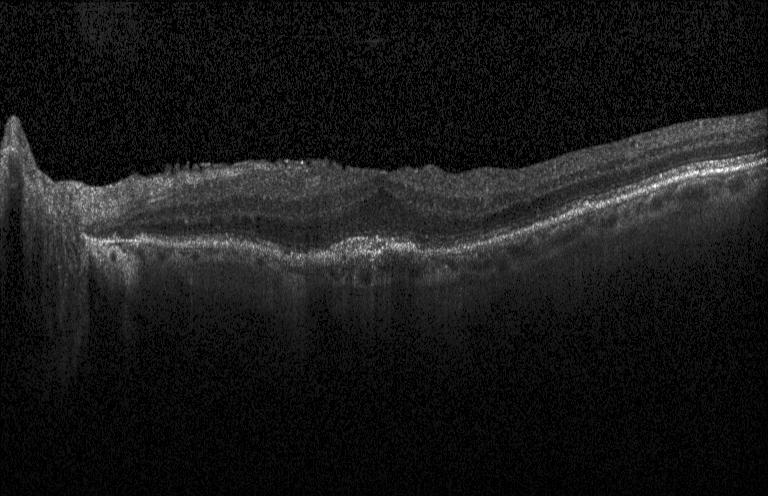

Optical coherence tomography B-scan; SD-OCT; macular scan; Heidelberg Spectralis
This B-scan demonstrates a choroidal neovascular membrane.